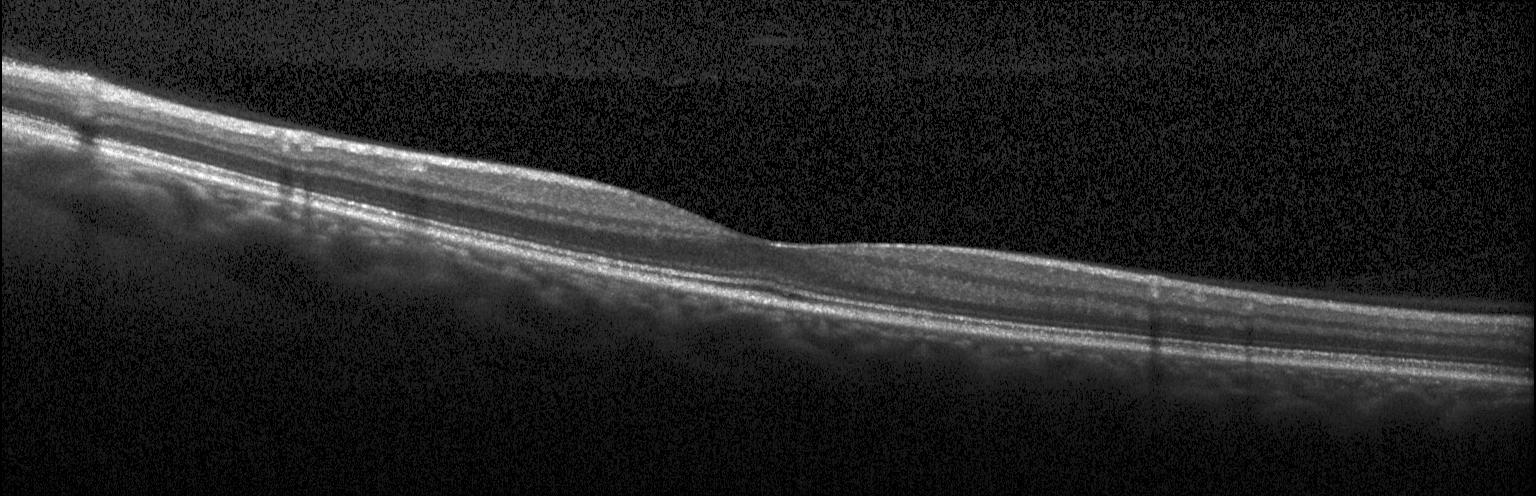

Dx: no choroidal neovascularization, no diabetic macular edema, and no drusen.